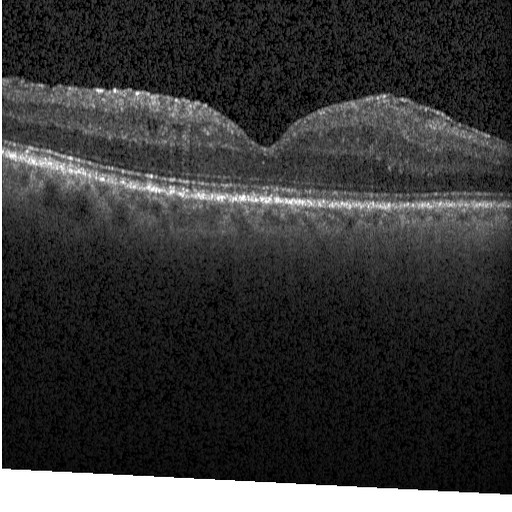
SD-OCT; retinal OCT B-scan; centered on the fovea; acquired on a Heidelberg Spectralis — Finding: DME.